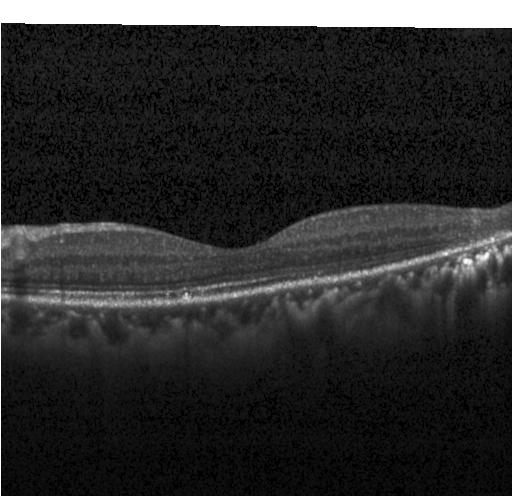

Heidelberg Spectralis OCT system · macular scan · retinal OCT B-scan. Finding: no CNV, no DME, and no drusen.